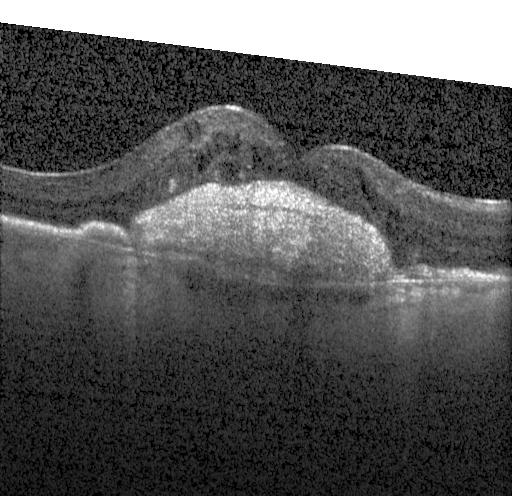

Retinal OCT cross-section, horizontal scan through the fovea, spectral-domain OCT. The scan shows CNV.